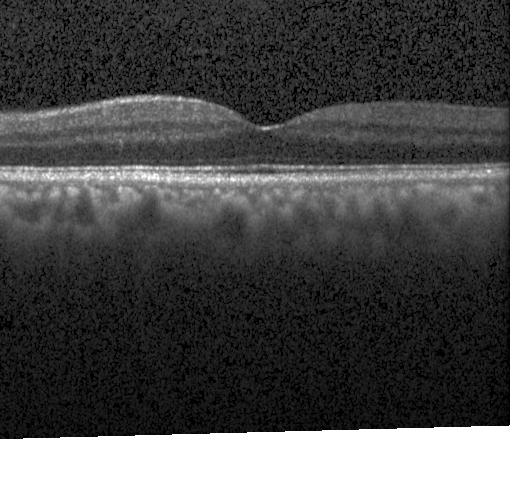
OCT B-scan showing no evidence of choroidal neovascularization, diabetic macular edema, or drusen.